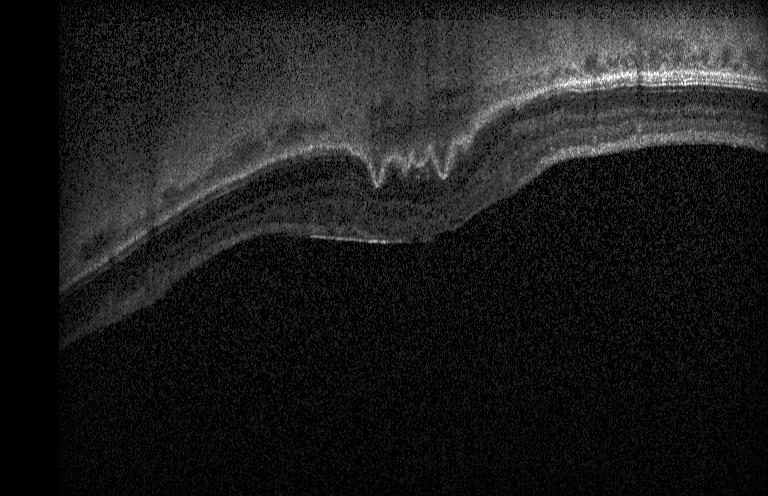
Macular OCT: a choroidal neovascular membrane.